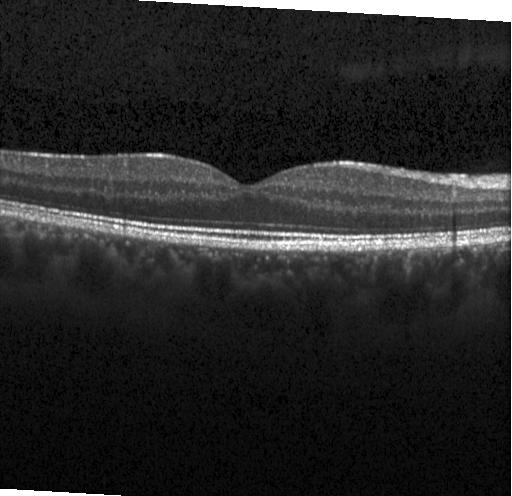
Macular OCT: neither choroidal neovascularization, diabetic macular edema, nor drusen.